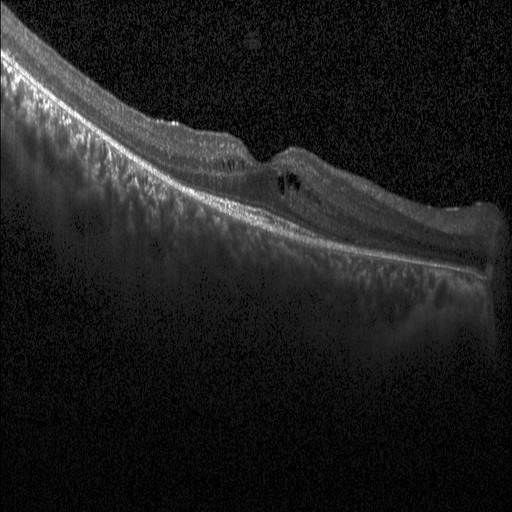

OCT line scan — This B-scan demonstrates diabetic macular edema (DME).